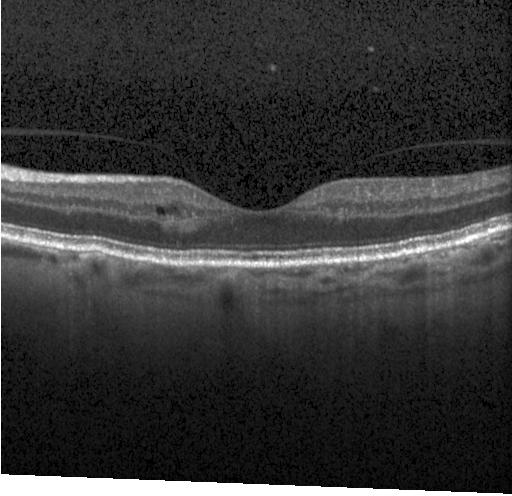
OCT finding: diabetic macular edema (DME).